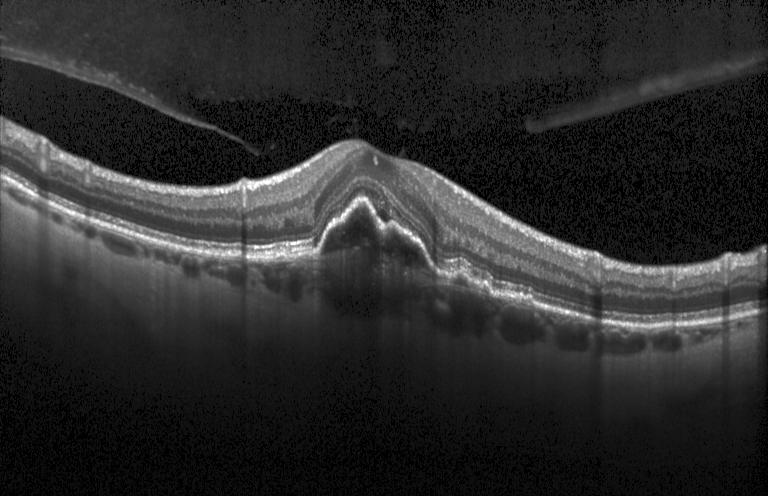 Centered on the fovea · retinal OCT cross-section · instrument: Heidelberg Spectralis · SD-OCT. The scan shows a choroidal neovascular membrane.